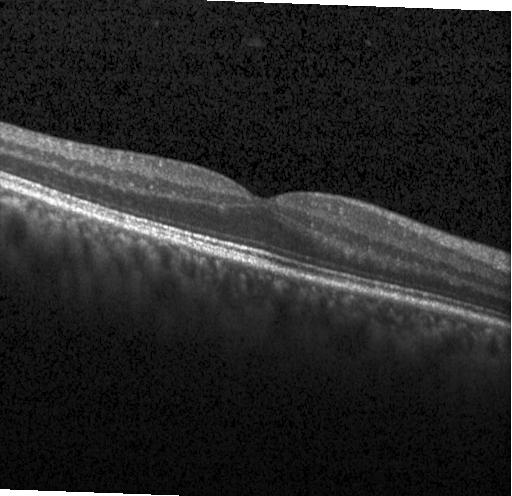

Heidelberg Spectralis. Optical coherence tomography scan
This B-scan demonstrates neither choroidal neovascularization, diabetic macular edema, nor drusen.